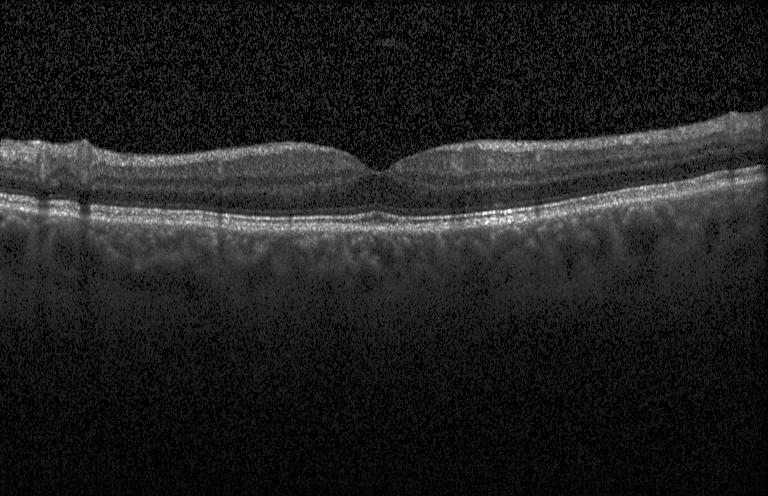
OCT line scan, spectral-domain OCT, horizontal scan through the fovea.
Finding: no choroidal neovascularization, no diabetic macular edema, and no drusen.